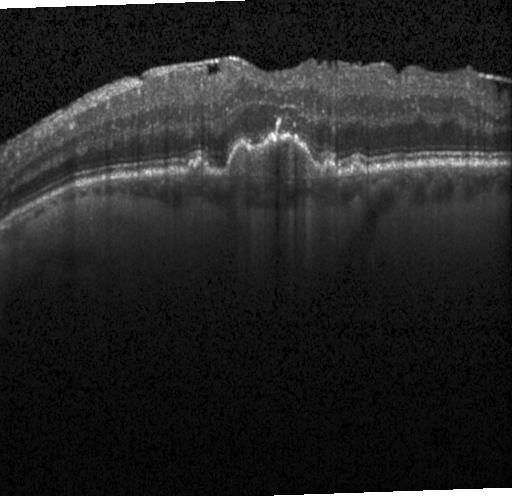

SD-OCT; retinal OCT B-scan. This B-scan demonstrates CNV.